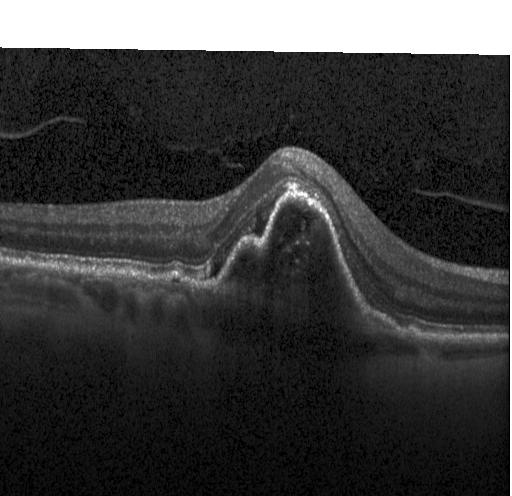

Retinal OCT cross-section. Heidelberg Spectralis OCT system. Macular scan. Spectral-domain OCT — Impression: choroidal neovascularization.